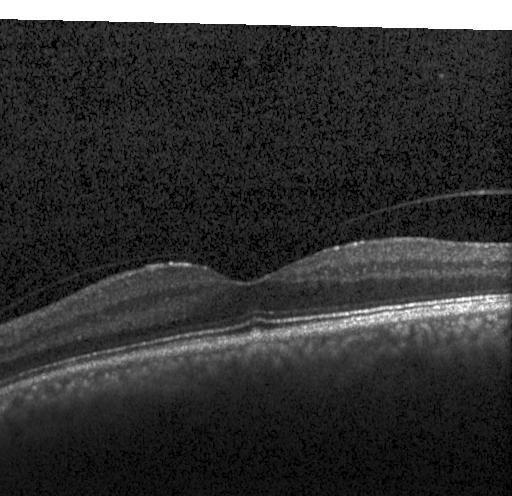 OCT line scan · SD-OCT · centered on the fovea. No choroidal neovascularization, diabetic macular edema, or drusen.